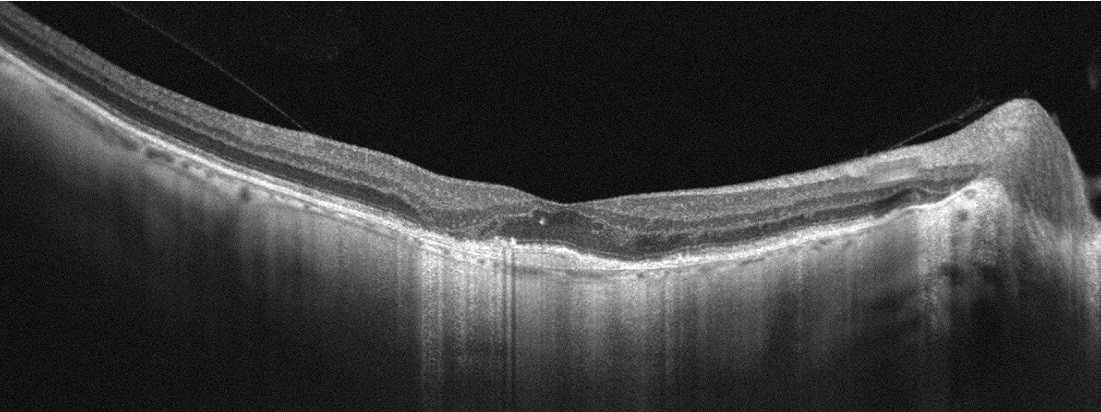

Macular scan; optical coherence tomography B-scan — Assessment: AMD.